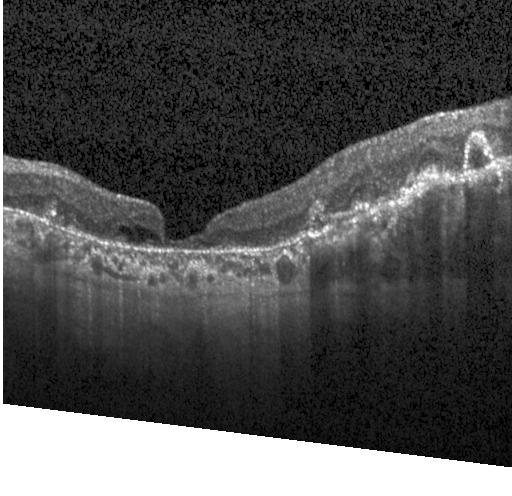

OCT B-scan; acquired on a Heidelberg Spectralis.
Dx: a choroidal neovascular membrane.